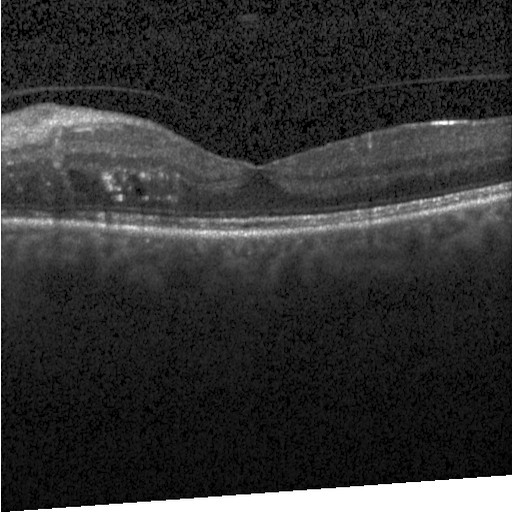 Retinal OCT cross-section showing DME.